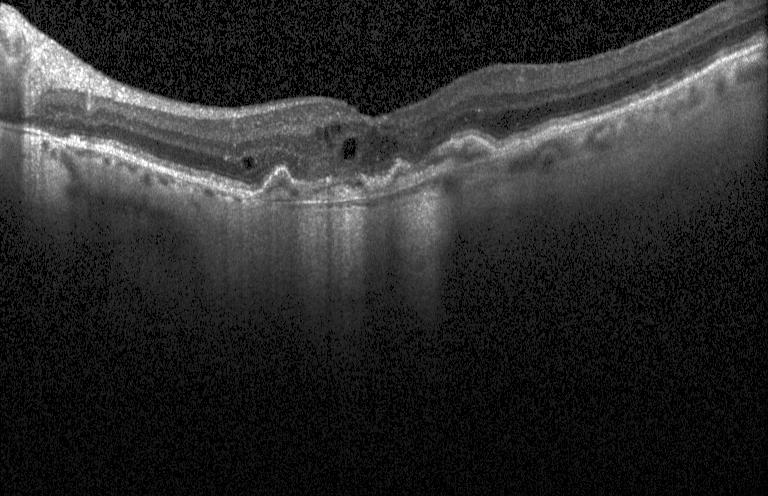

Impression: choroidal neovascularization (CNV).